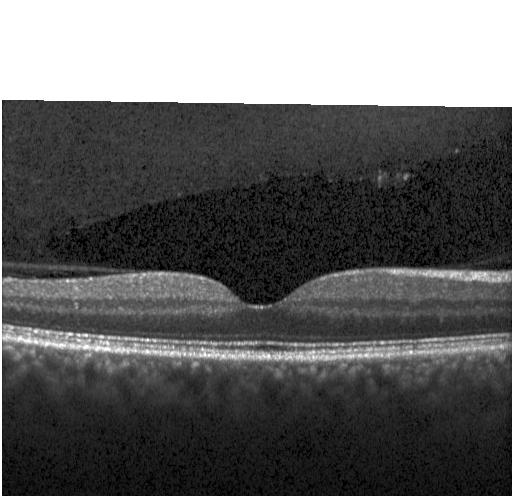
Dx: no choroidal neovascularization, no diabetic macular edema, and no drusen.